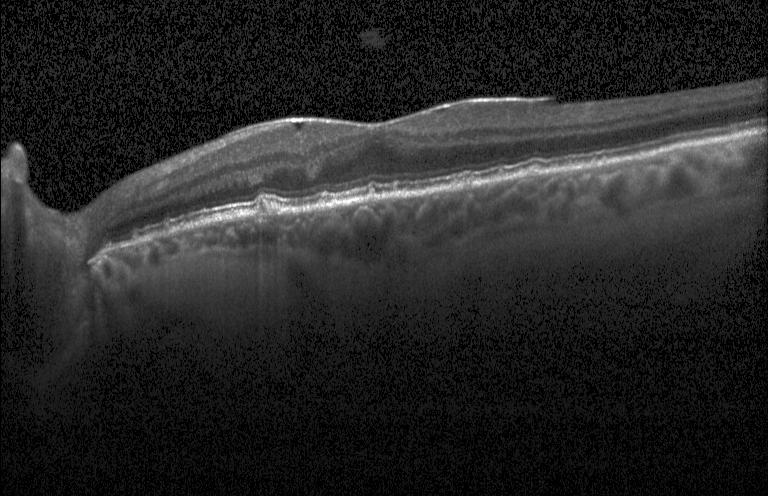

Retinal OCT cross-section
Impression: multiple drusen.